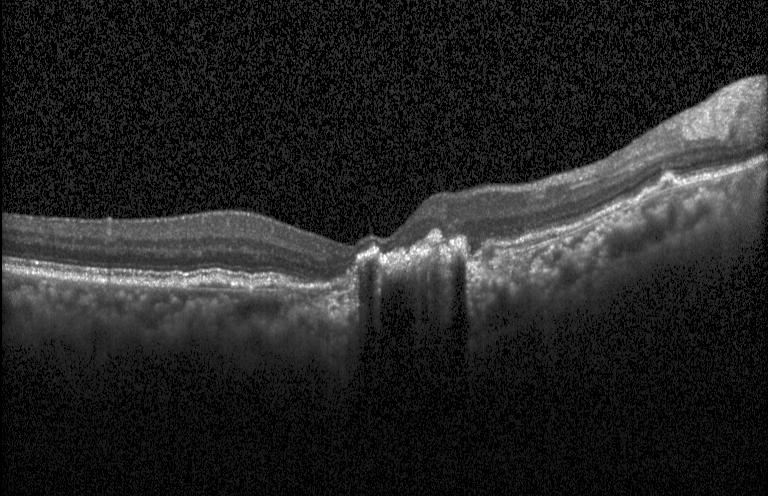

Macular OCT demonstrating a choroidal neovascular membrane.